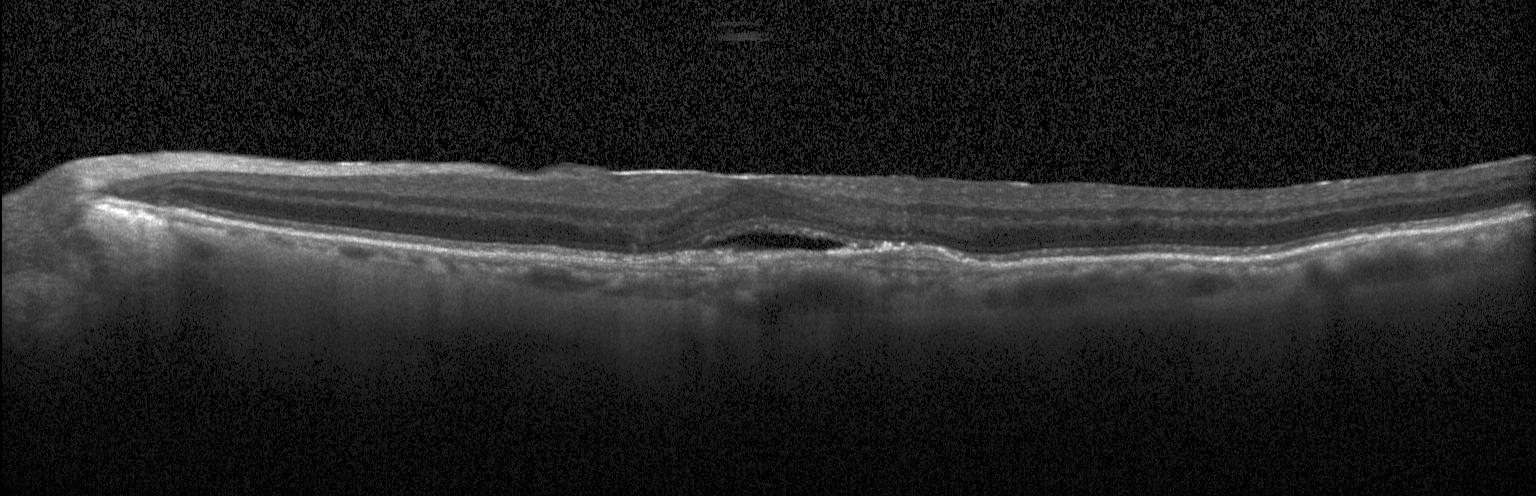

Retinal OCT B-scan; instrument: Heidelberg Spectralis; through the macula.
Macular OCT: a choroidal neovascular membrane.